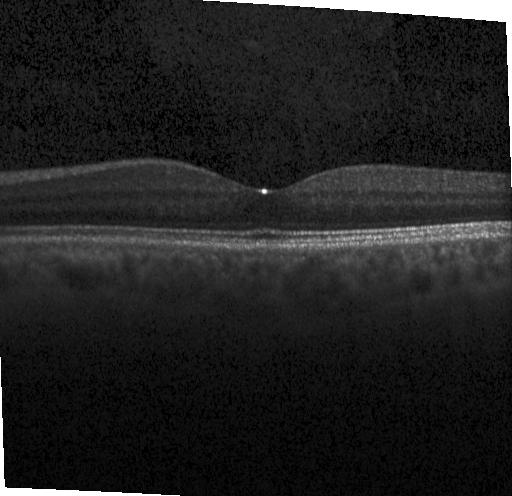 Macular scan. OCT B-scan.
Assessment: no choroidal neovascularization, diabetic macular edema, or drusen.